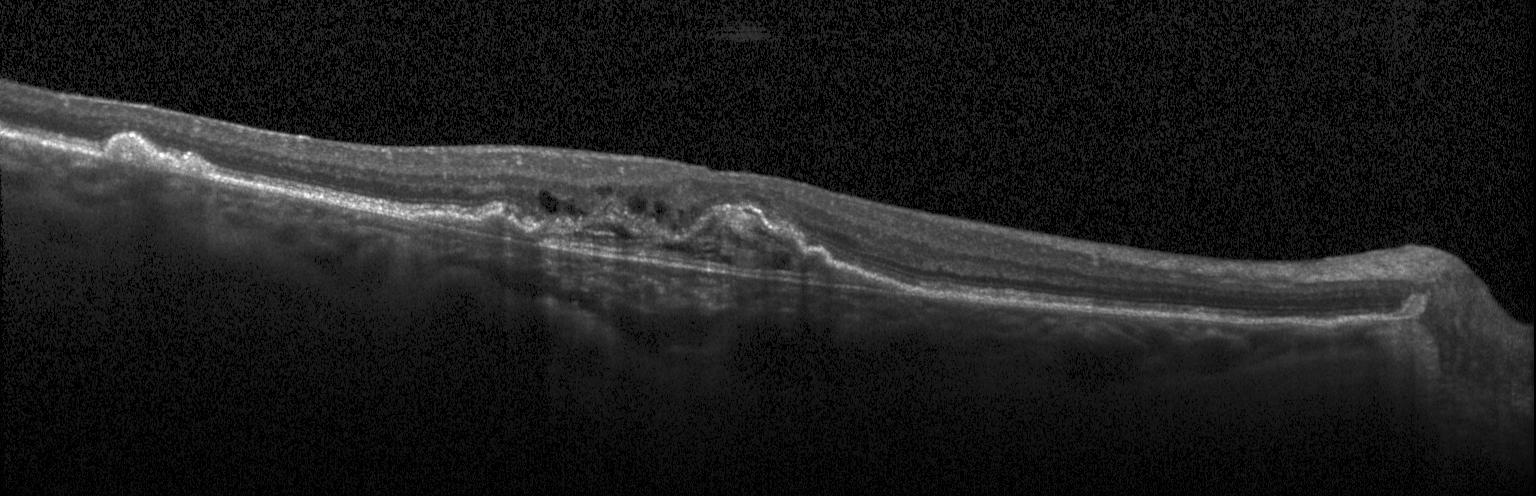
Finding: a choroidal neovascular membrane.